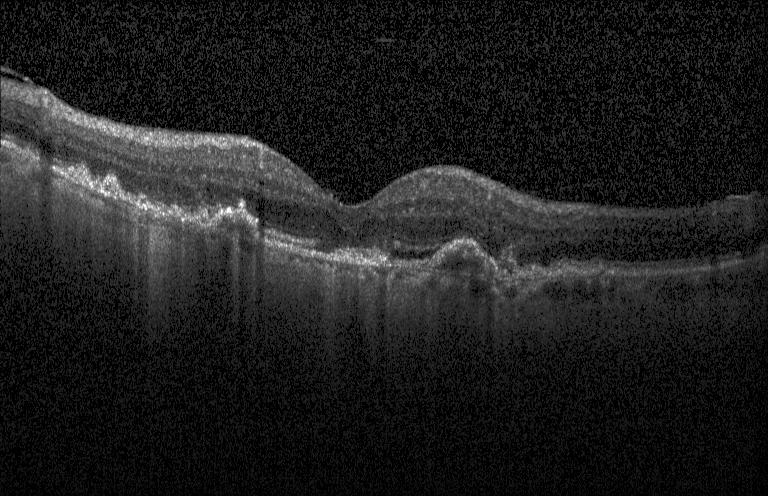 Spectral-domain OCT B-scan: a choroidal neovascular membrane.